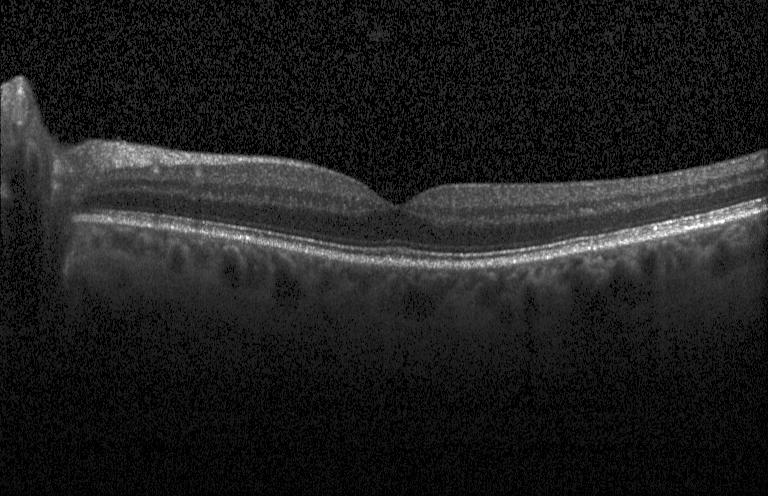

Retinal OCT cross-section; spectral-domain optical coherence tomography
Diagnosis: no evidence of choroidal neovascularization, diabetic macular edema, or drusen.